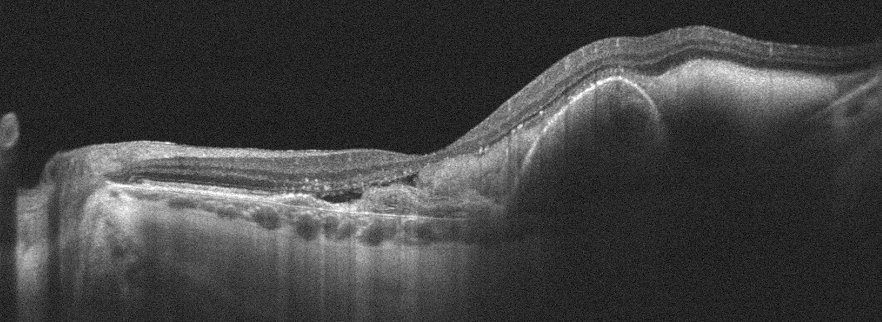

Retinal OCT cross-section, instrument: Optovue Avanti RTVue XR, left eye. Dx: age-related macular degeneration (AMD).